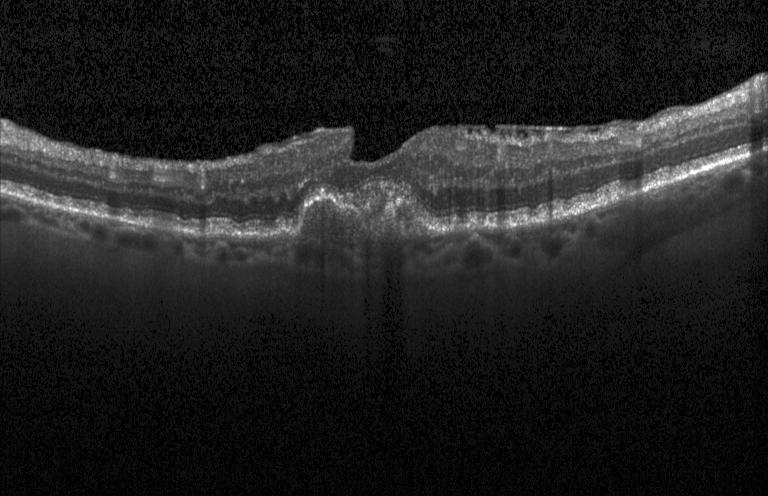

SD-OCT; acquired on a Heidelberg Spectralis; retinal OCT cross-section — OCT finding: a choroidal neovascular membrane.